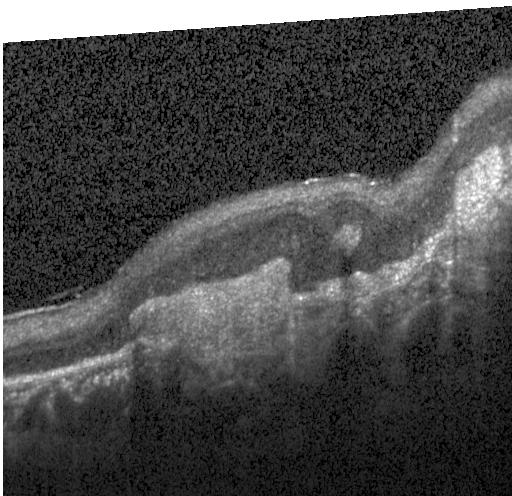 Impression: a choroidal neovascular membrane.